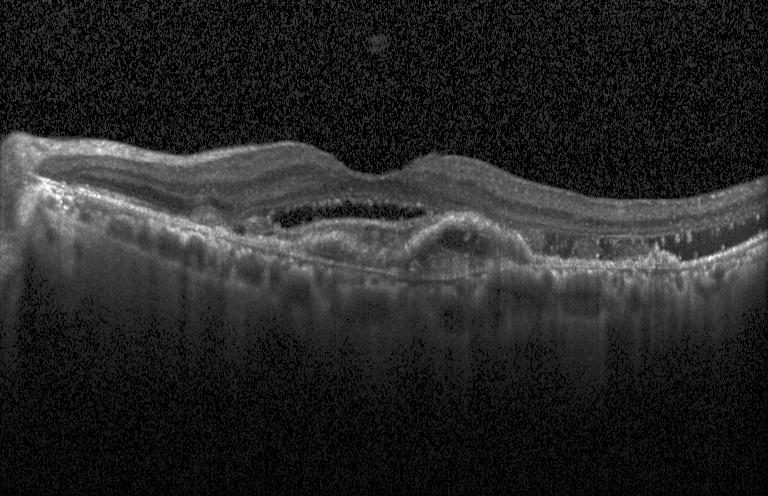
Through the macula; spectral-domain OCT; Heidelberg Spectralis; retinal OCT B-scan.
The scan shows choroidal neovascularization (CNV).